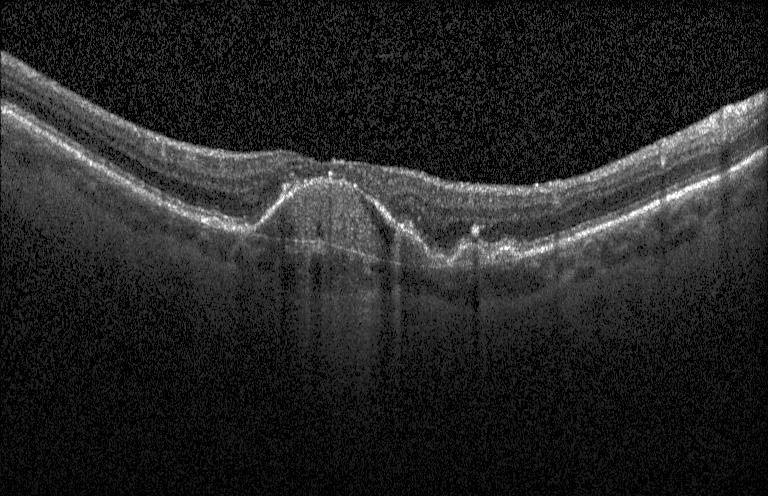 Macular scan · OCT B-scan — Impression: choroidal neovascularization (CNV).